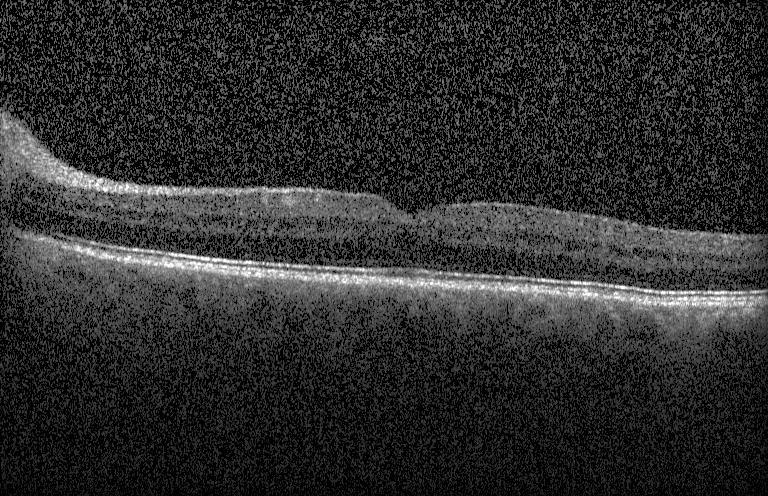

Spectral-domain OCT B-scan: no choroidal neovascularization, no diabetic macular edema, and no drusen.